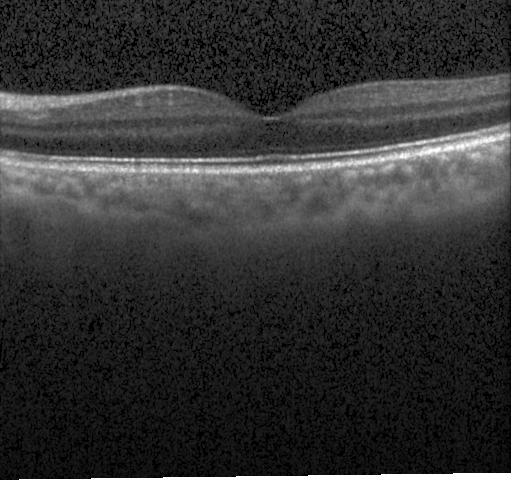 OCT B-scan showing no evidence of choroidal neovascularization, diabetic macular edema, or drusen.